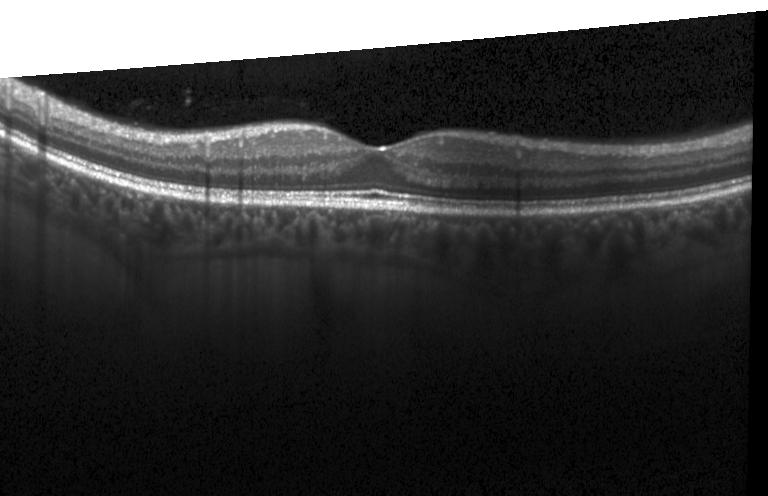 Diagnosis: no choroidal neovascularization, no diabetic macular edema, and no drusen.